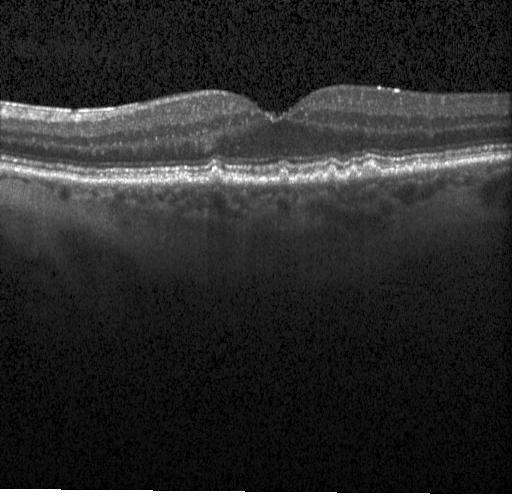
OCT line scan
This B-scan demonstrates multiple drusen.